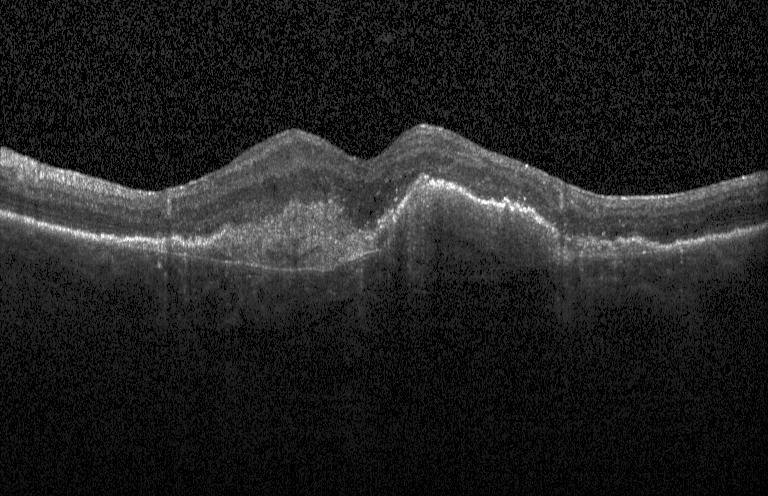 Retinal OCT cross-section showing a choroidal neovascular membrane.